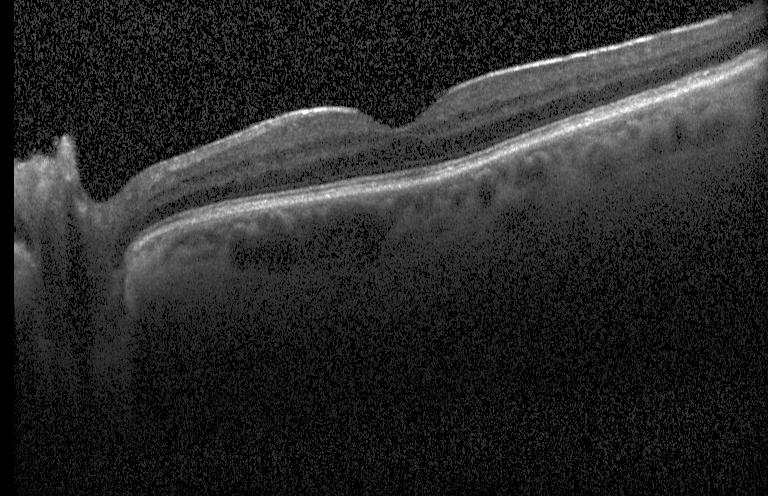 Optical coherence tomography B-scan — This B-scan demonstrates no choroidal neovascularization, diabetic macular edema, or drusen.